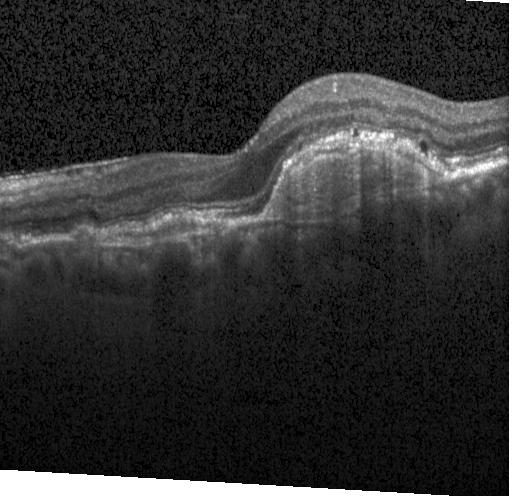
Retinal OCT cross-section showing CNV.